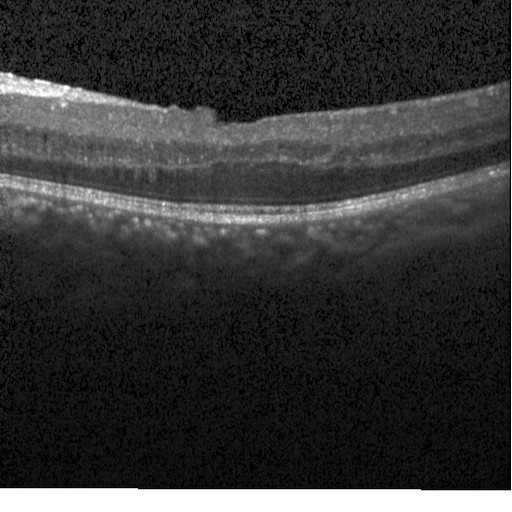
Retinal OCT B-scan; centered on the fovea; spectral-domain optical coherence tomography
Assessment: diabetic macular edema.